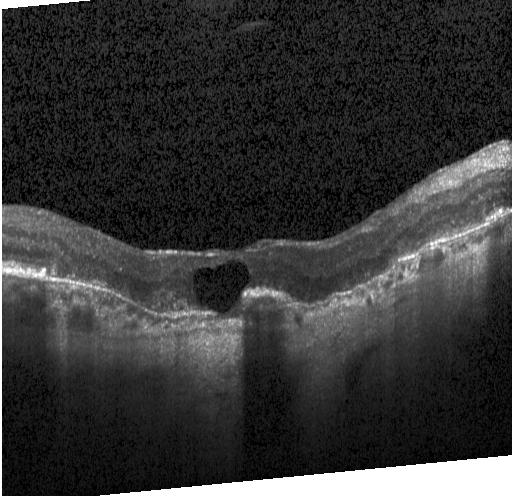
Optical coherence tomography scan. Acquired on a Heidelberg Spectralis. A choroidal neovascular membrane.